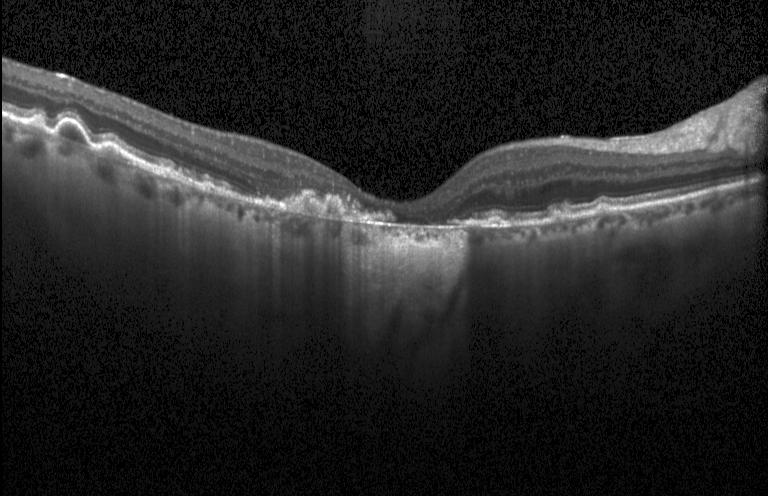
OCT B-scan
Diagnosis: choroidal neovascularization.